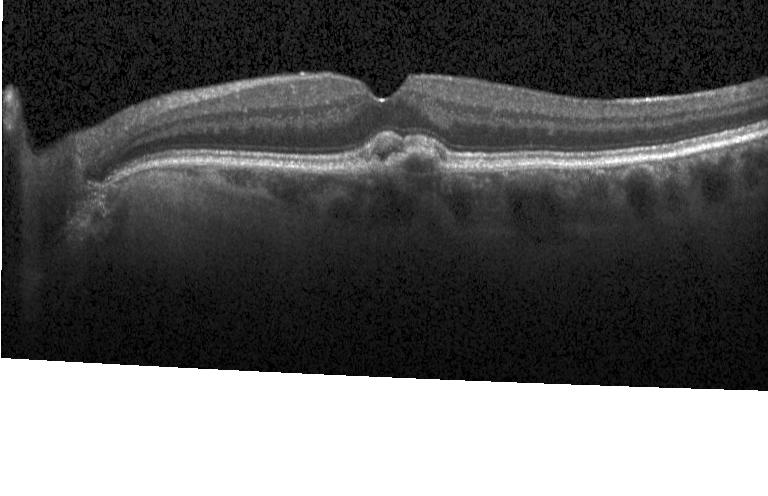

The scan shows choroidal neovascularization.